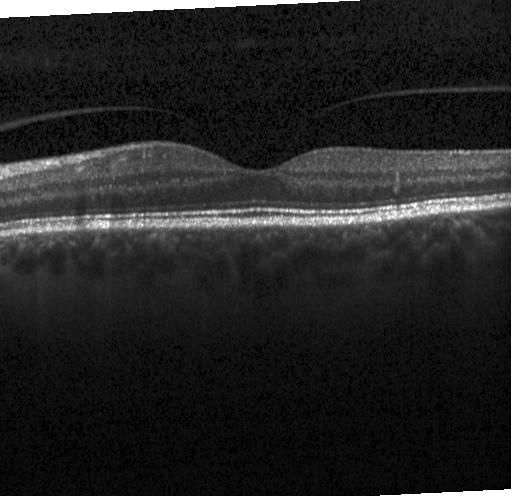
Assessment: no evidence of choroidal neovascularization, diabetic macular edema, or drusen.